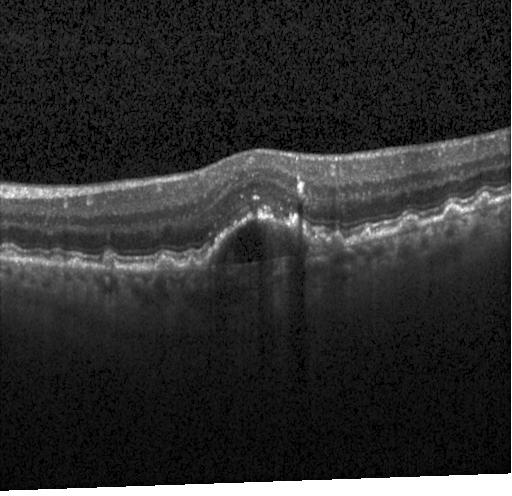
Retinal OCT cross-section. Spectral-domain OCT — Assessment: a choroidal neovascular membrane.